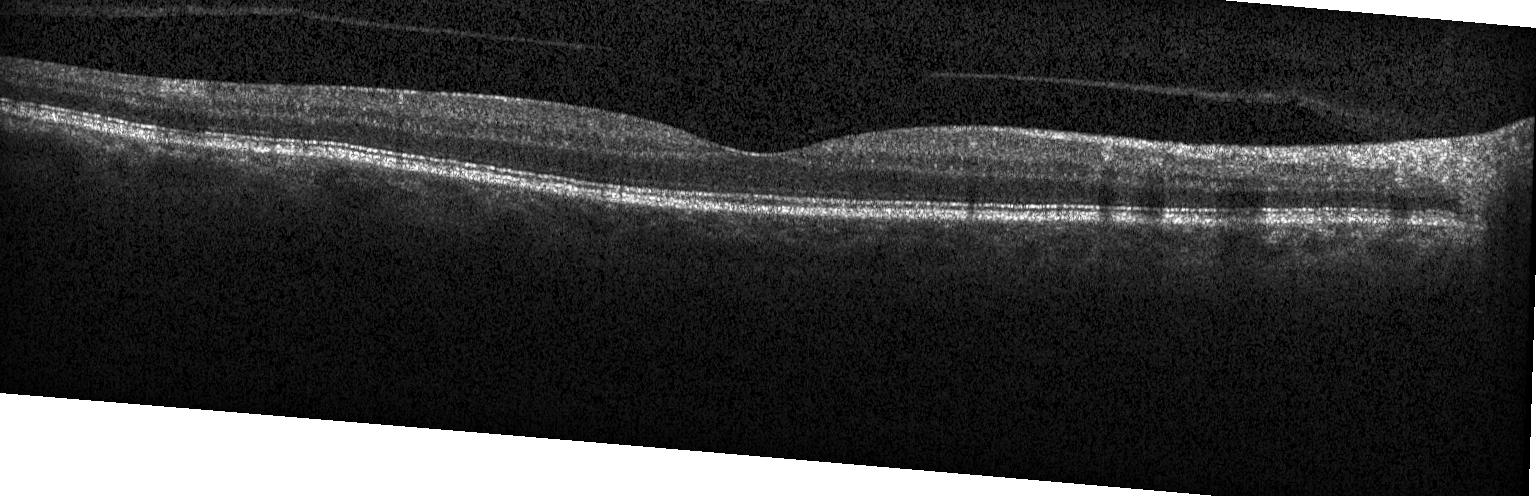
Impression: no CNV, no DME, and no drusen.